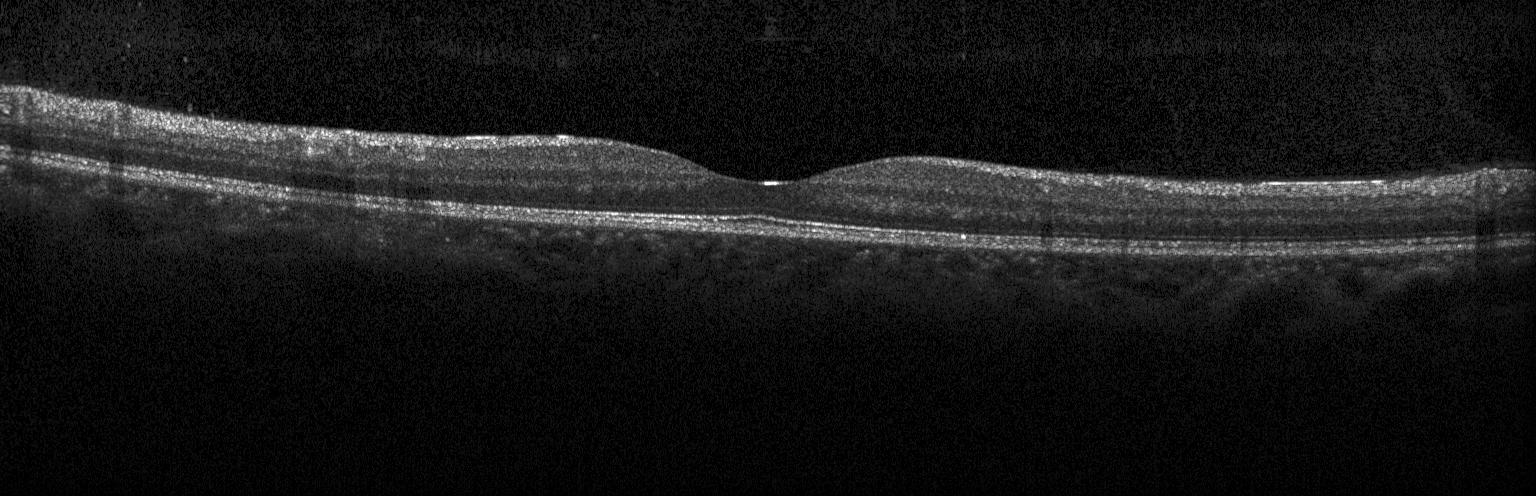

Macular OCT: no evidence of choroidal neovascularization, diabetic macular edema, or drusen.